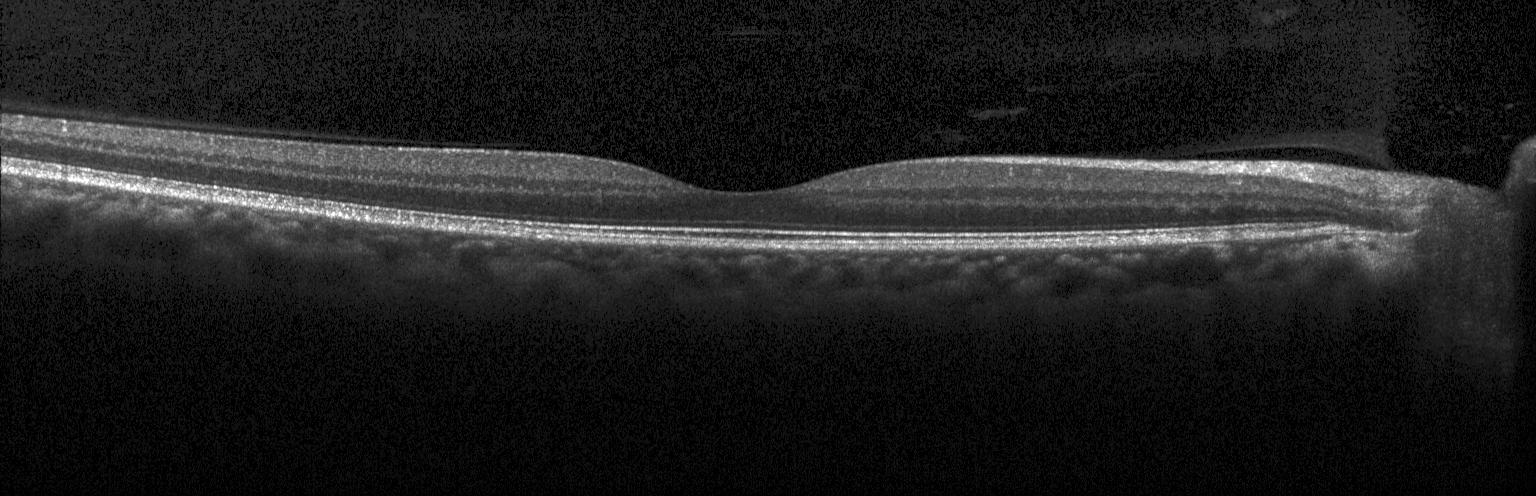

Centered on the fovea · retinal OCT B-scan · spectral-domain OCT · instrument: Heidelberg Spectralis — Finding: no evidence of choroidal neovascularization, diabetic macular edema, or drusen.